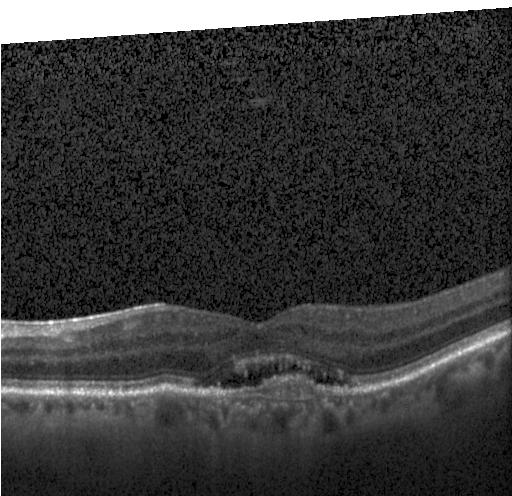 Fovea-centered · Heidelberg Spectralis OCT system · spectral-domain OCT · OCT B-scan — Diagnosis: choroidal neovascularization.